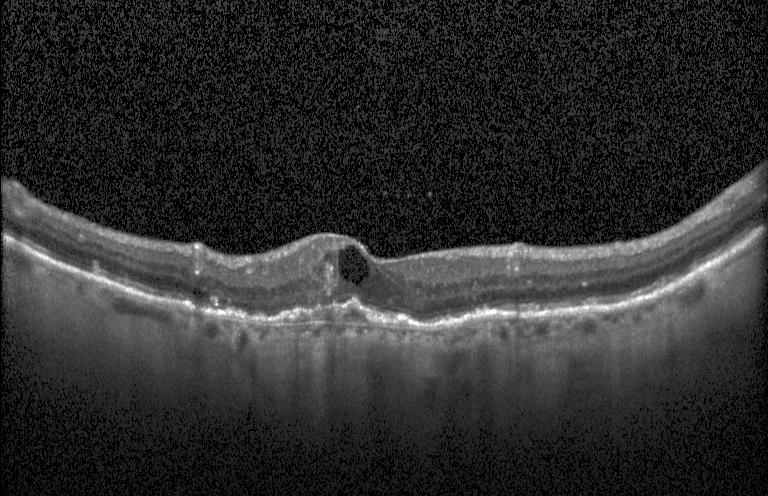

Instrument: Heidelberg Spectralis · spectral-domain optical coherence tomography · centered on the fovea · optical coherence tomography B-scan
A choroidal neovascular membrane.